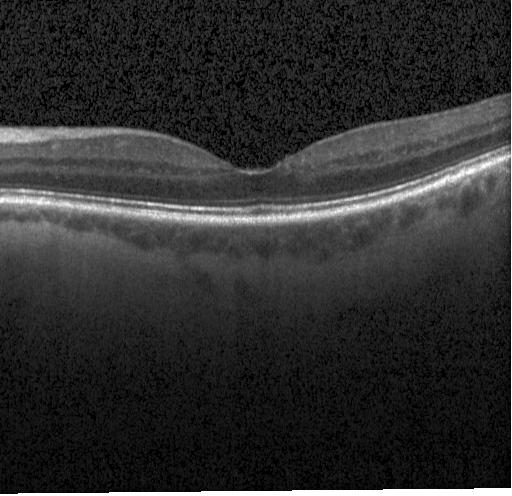

Spectral-domain OCT B-scan: no choroidal neovascularization, no diabetic macular edema, and no drusen.